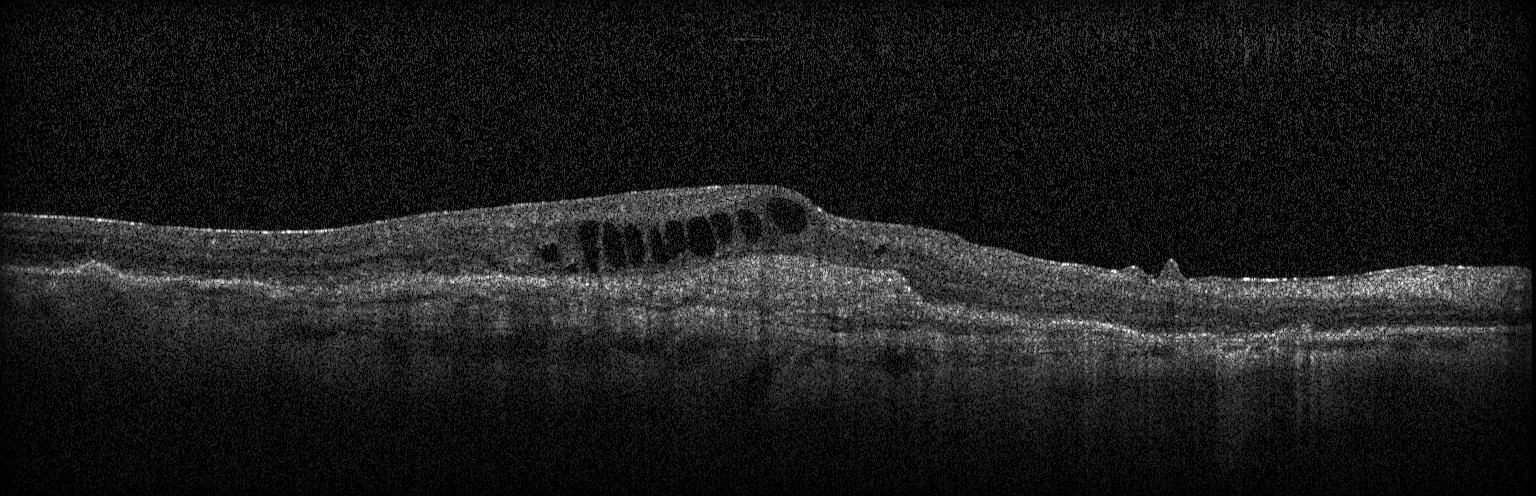

Diagnosis: CNV.